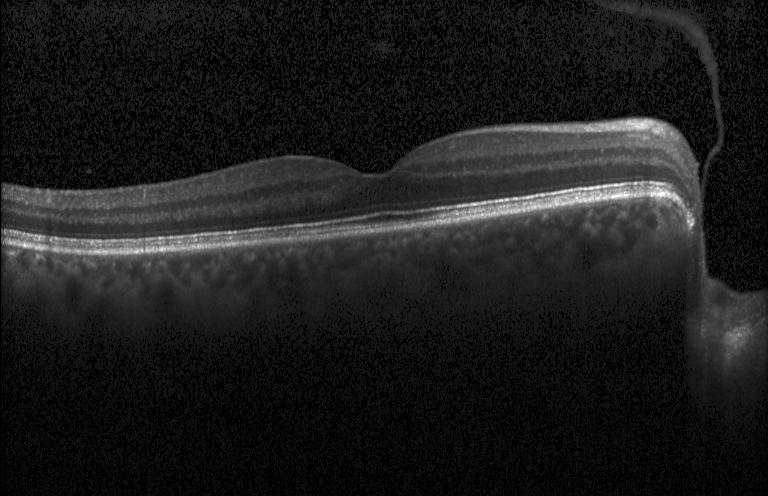 OCT B-scan · through the macula · spectral-domain optical coherence tomography · Heidelberg Spectralis OCT system — Impression: no evidence of CNV, DME, or drusen.